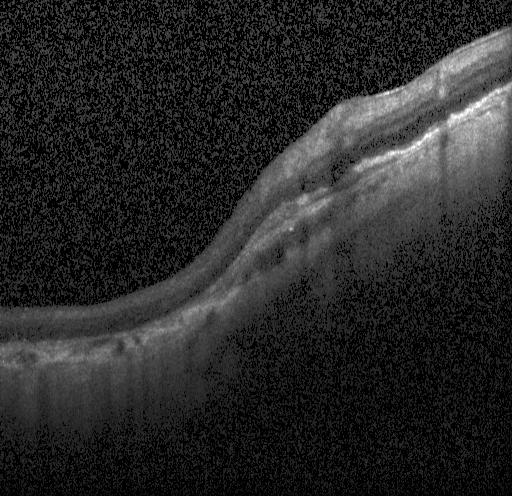

Acquired on a Heidelberg Spectralis, retinal OCT B-scan — Impression: choroidal neovascularization.